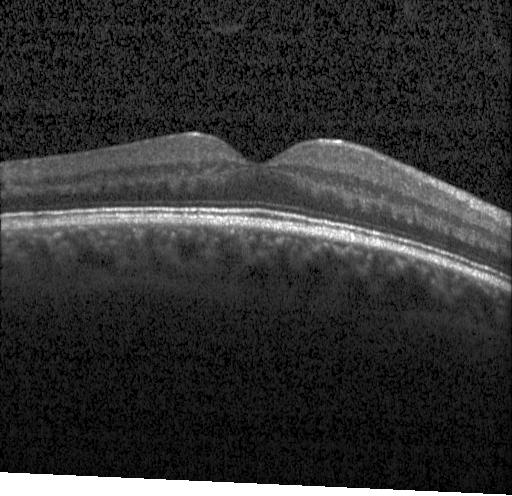

Macular scan; optical coherence tomography B-scan.
Impression: no choroidal neovascularization, no diabetic macular edema, and no drusen.